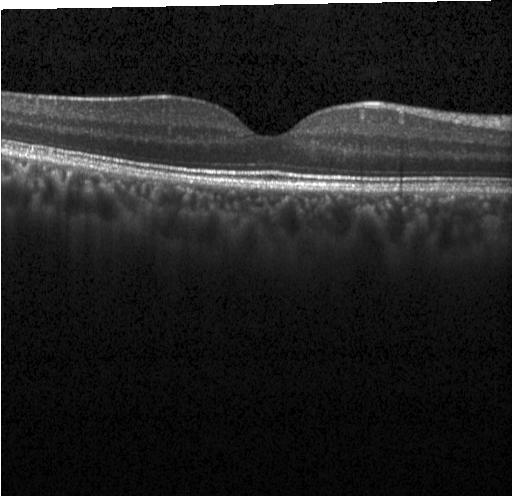 Through the macula. Retinal OCT cross-section. Instrument: Heidelberg Spectralis. SD-OCT
Diagnosis: no CNV, DME, or drusen.